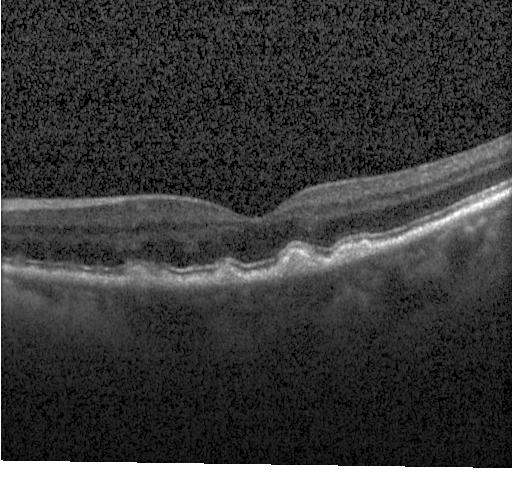 OCT line scan; centered on the fovea; spectral-domain optical coherence tomography; instrument: Heidelberg Spectralis. Macular OCT: drusen.